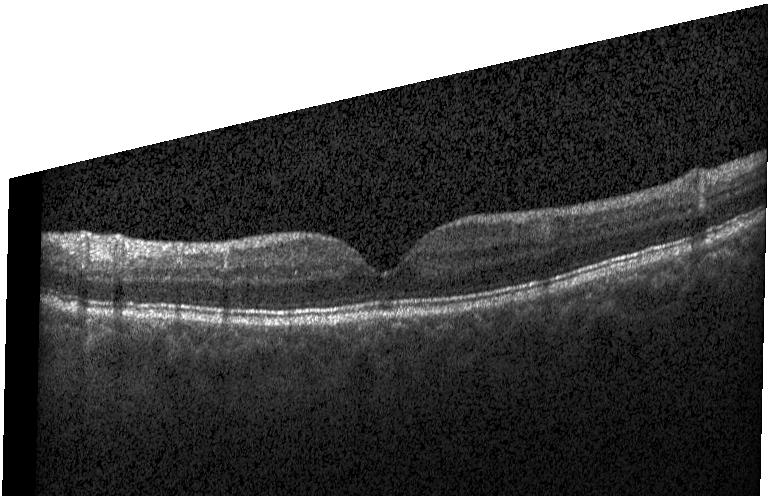 Horizontal scan through the fovea; optical coherence tomography scan; instrument: Heidelberg Spectralis
Diagnosis: no choroidal neovascularization, diabetic macular edema, or drusen.